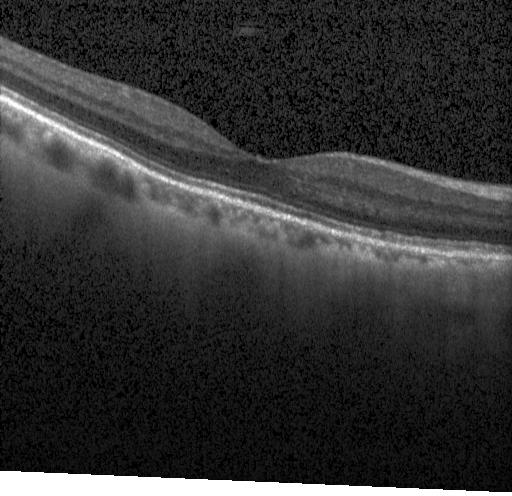

Spectral-domain OCT B-scan: no choroidal neovascularization, diabetic macular edema, or drusen.